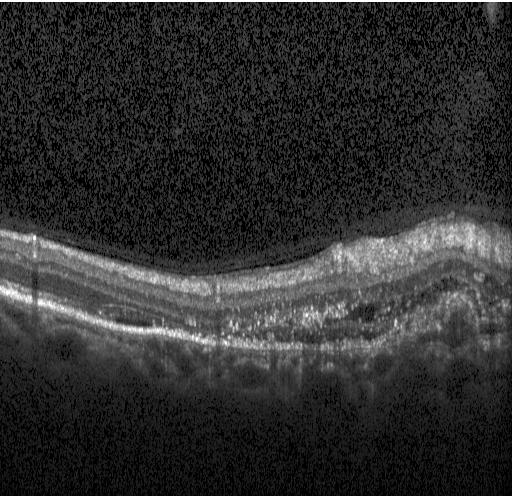

Macular OCT: a choroidal neovascular membrane.